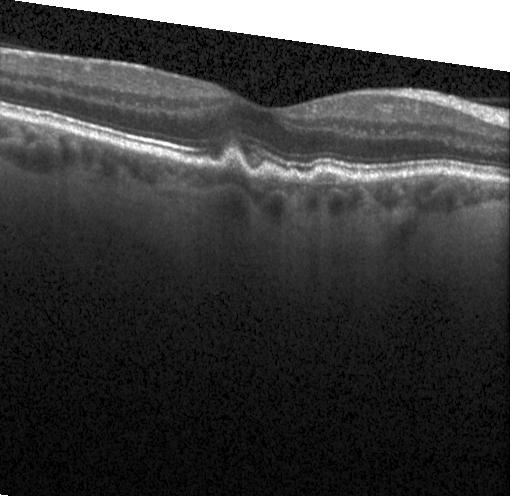

Instrument: Heidelberg Spectralis. SD-OCT. Optical coherence tomography scan. Macular scan. OCT finding: multiple drusen.